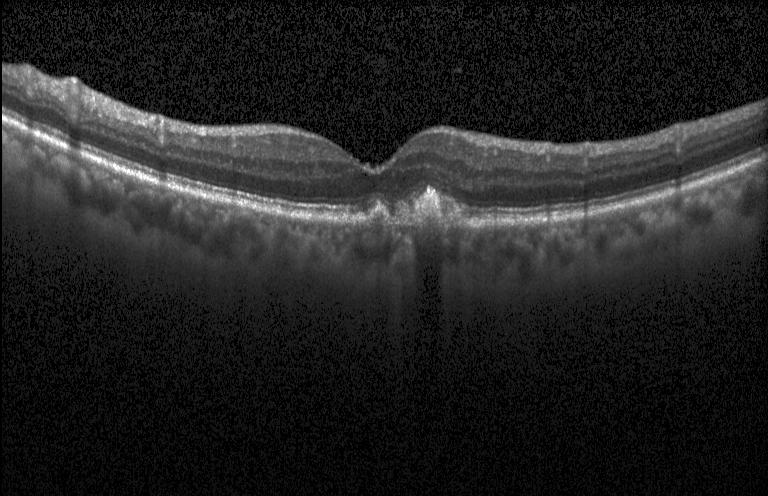
Heidelberg Spectralis OCT system; SD-OCT; optical coherence tomography scan; macular scan
This B-scan demonstrates multiple drusen.